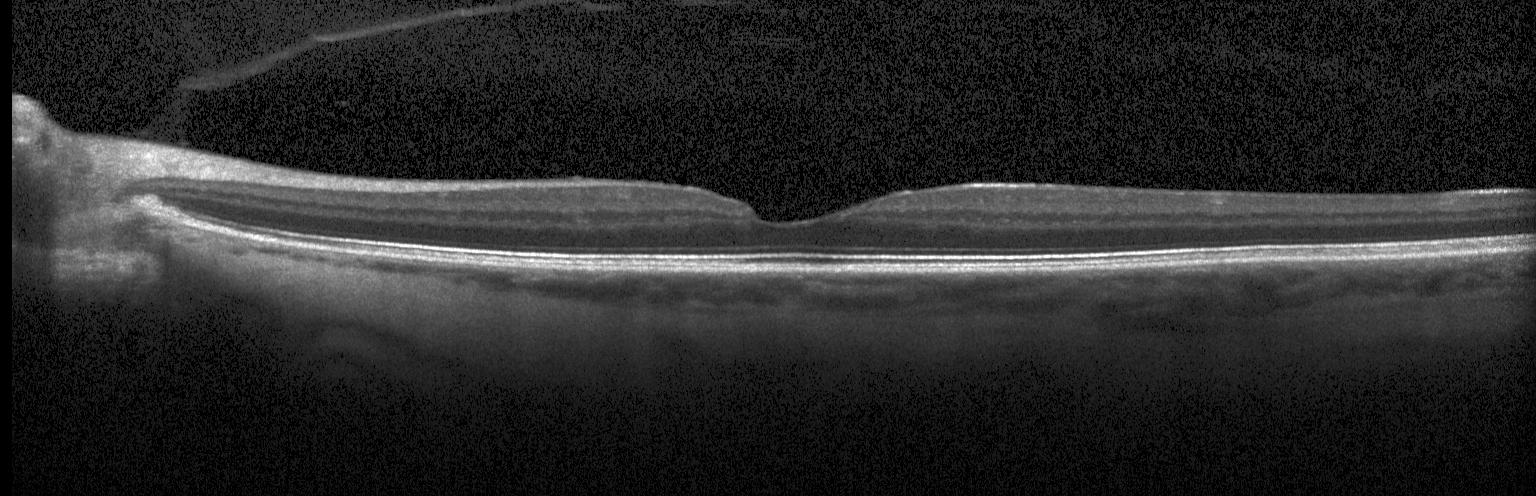
OCT line scan. OCT finding: no choroidal neovascularization, no diabetic macular edema, and no drusen.